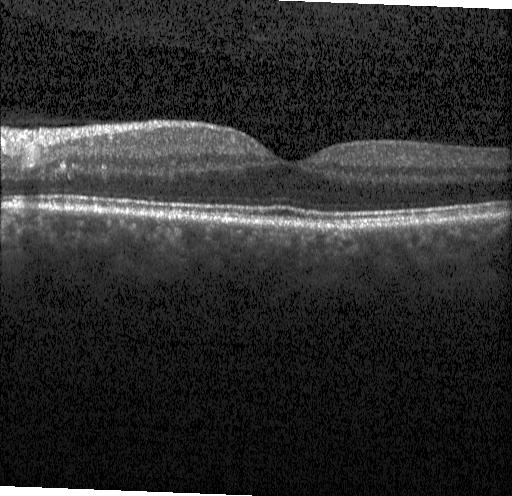
Macular OCT: no choroidal neovascularization, no diabetic macular edema, and no drusen.